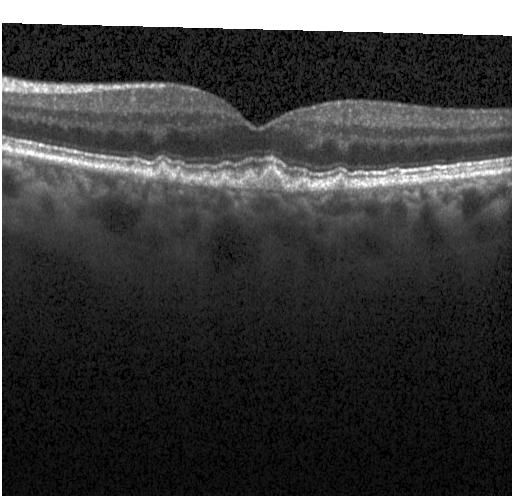
Optical coherence tomography scan. Finding: multiple drusen.